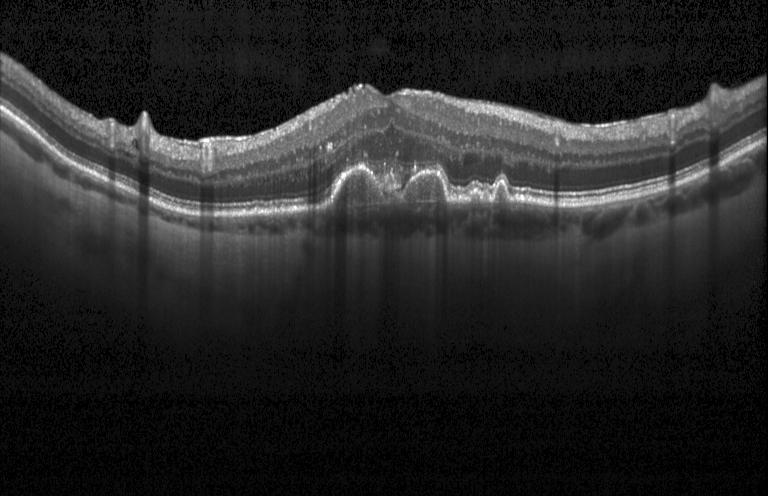 Impression: multiple drusen.